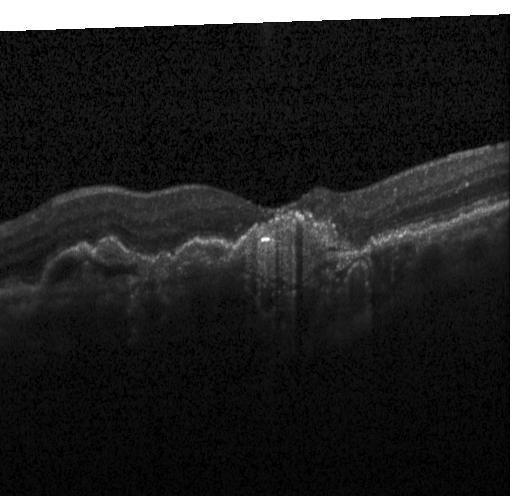 Macular OCT: choroidal neovascularization (CNV).